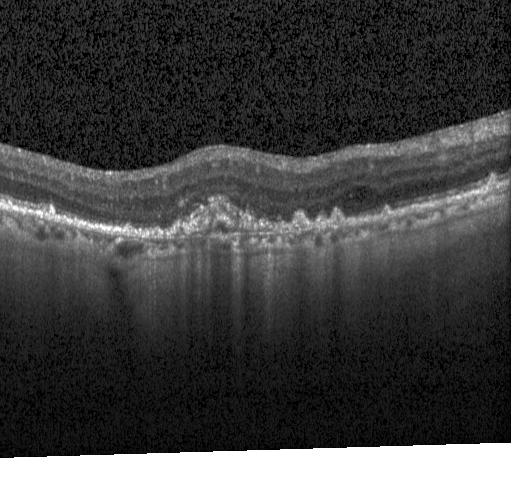
Heidelberg Spectralis OCT system, retinal OCT cross-section. This B-scan demonstrates a choroidal neovascular membrane.